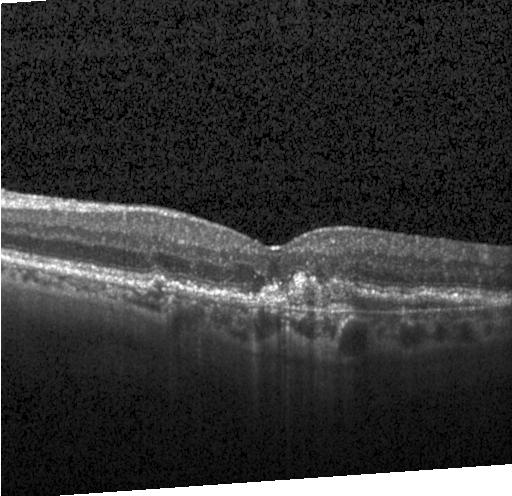 Optical coherence tomography B-scan · SD-OCT.
Finding: a choroidal neovascular membrane.